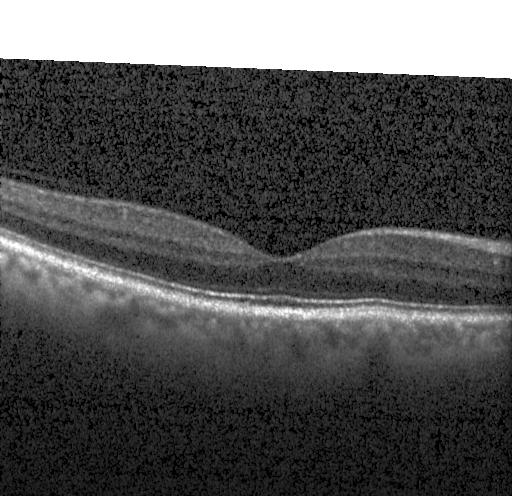
OCT B-scan
The scan shows no CNV, DME, or drusen.